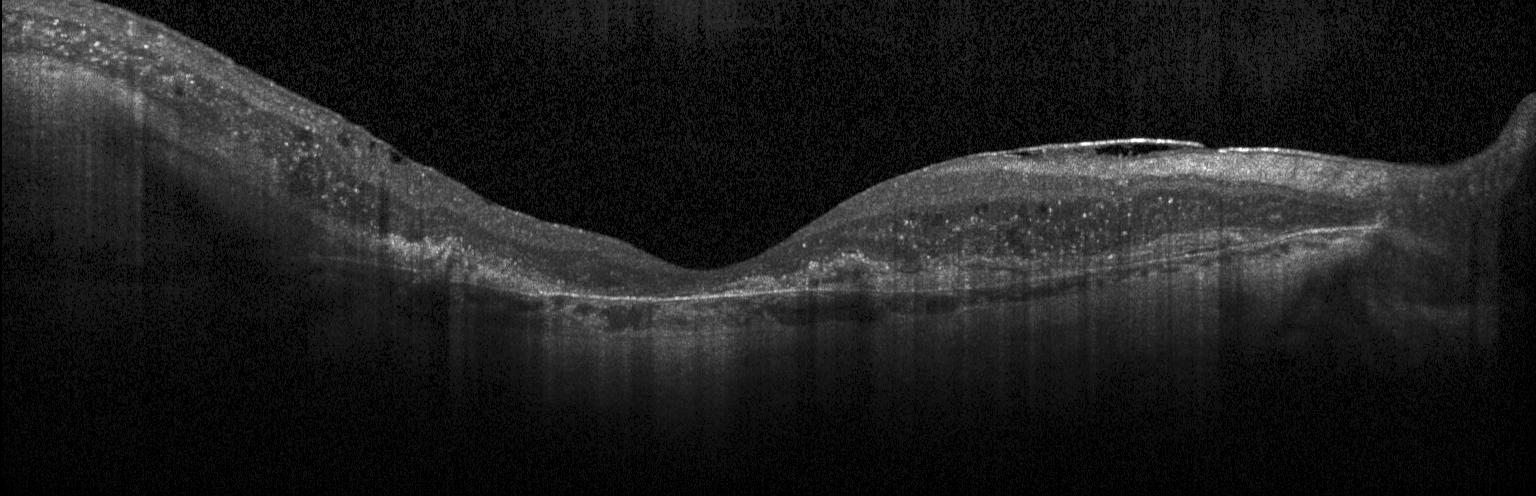
SD-OCT; OCT line scan; instrument: Heidelberg Spectralis
OCT finding: choroidal neovascularization (CNV).